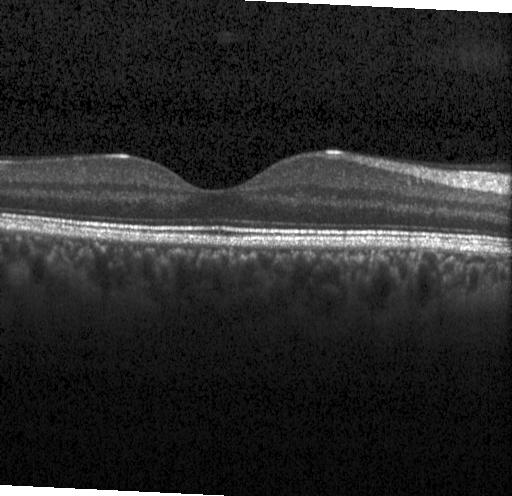 Heidelberg Spectralis OCT system; retinal OCT cross-section; spectral-domain OCT.
Diagnosis: neither choroidal neovascularization, diabetic macular edema, nor drusen.